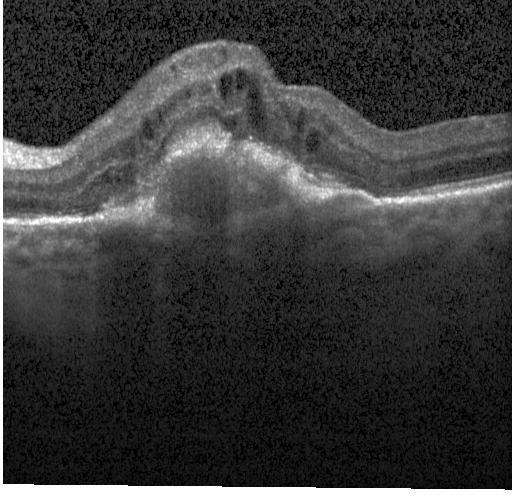 Macular OCT demonstrating a choroidal neovascular membrane.